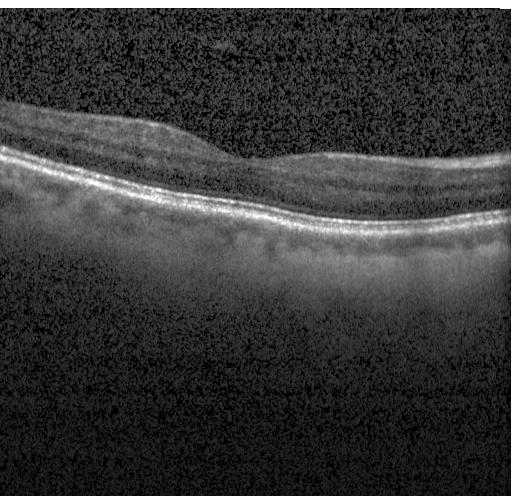
OCT line scan. Through the macula. SD-OCT. Acquired on a Heidelberg Spectralis
No CNV, no DME, and no drusen.